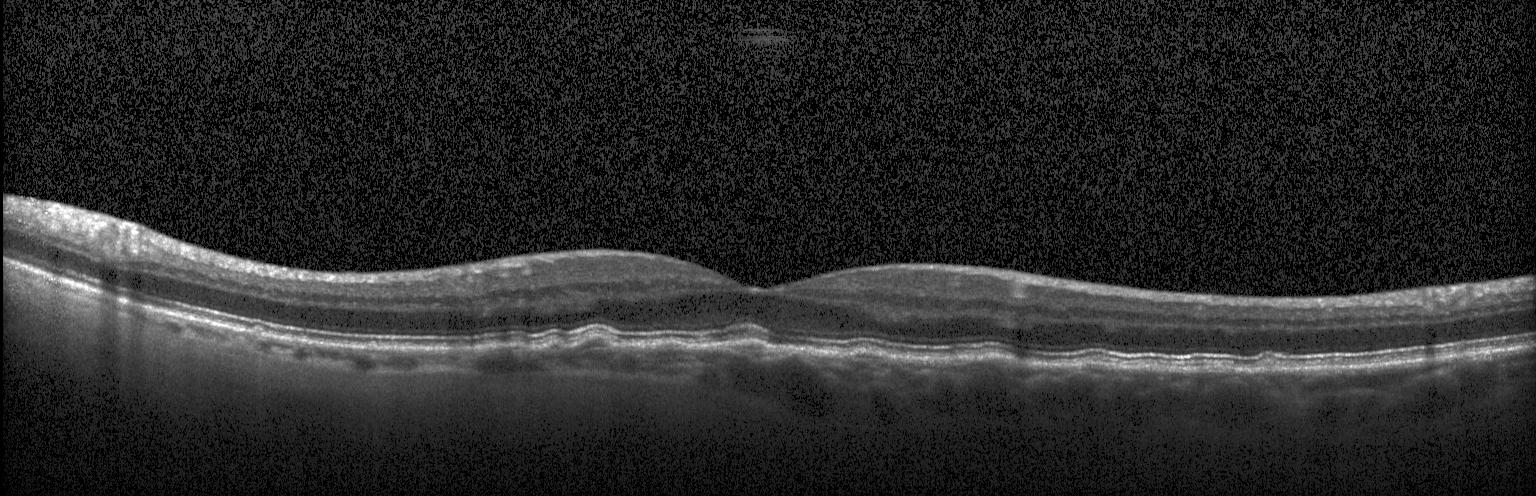

Macular OCT: multiple drusen.